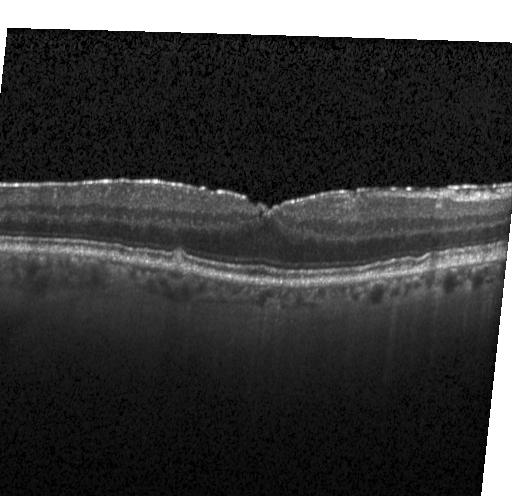
OCT B-scan
Finding: multiple drusen.